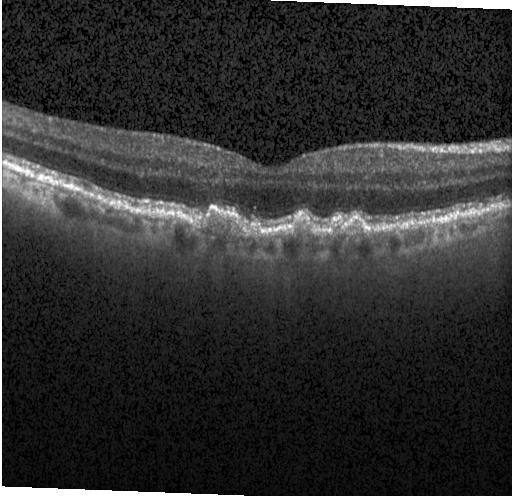

Spectral-domain OCT B-scan: drusen.